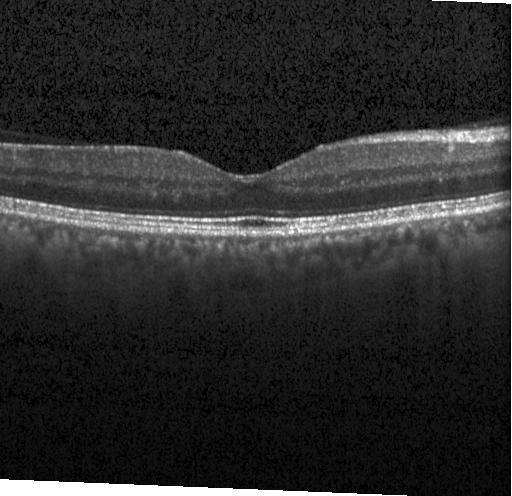 Optical coherence tomography scan, macular scan, spectral-domain OCT. The scan shows no choroidal neovascularization, no diabetic macular edema, and no drusen.